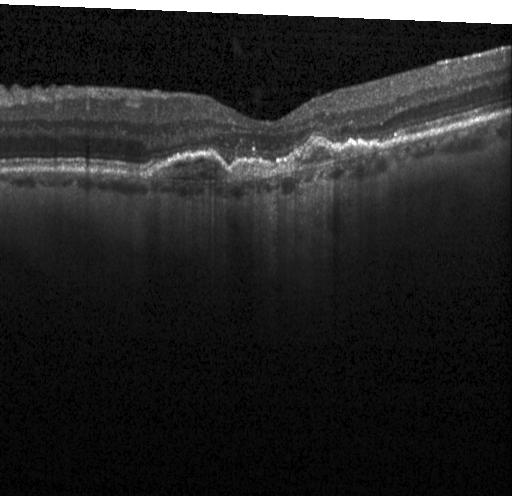 Optical coherence tomography B-scan, horizontal scan through the fovea, spectral-domain optical coherence tomography, acquired on a Heidelberg Spectralis — Finding: CNV.